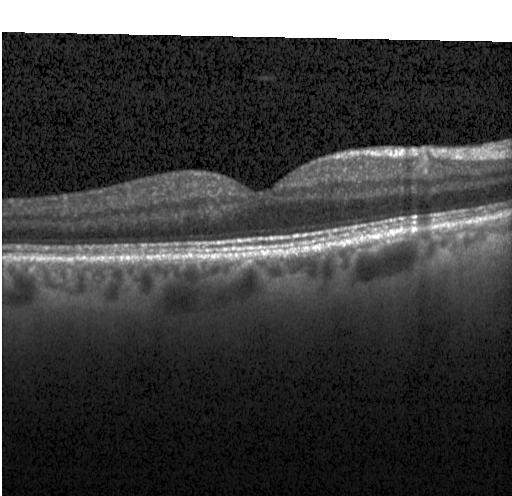
Dx: neither choroidal neovascularization, diabetic macular edema, nor drusen.